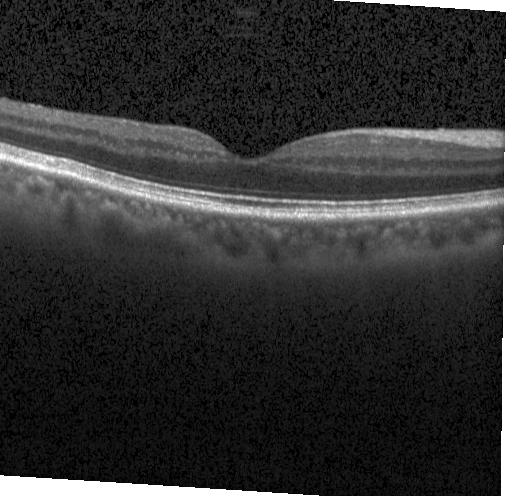 Impression: no choroidal neovascularization, no diabetic macular edema, and no drusen.